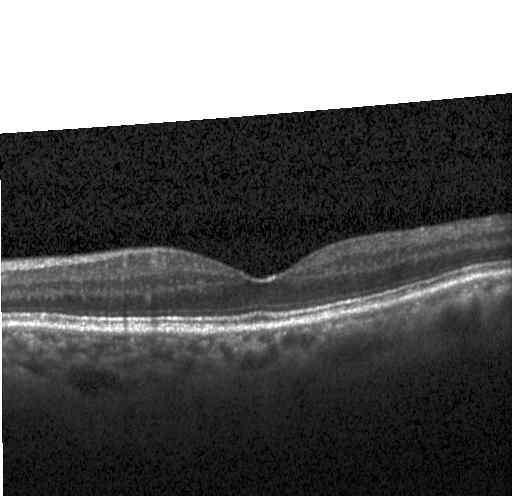
Through the macula, acquired on a Heidelberg Spectralis, SD-OCT, OCT B-scan. Diagnosis: neither CNV, DME, nor drusen.